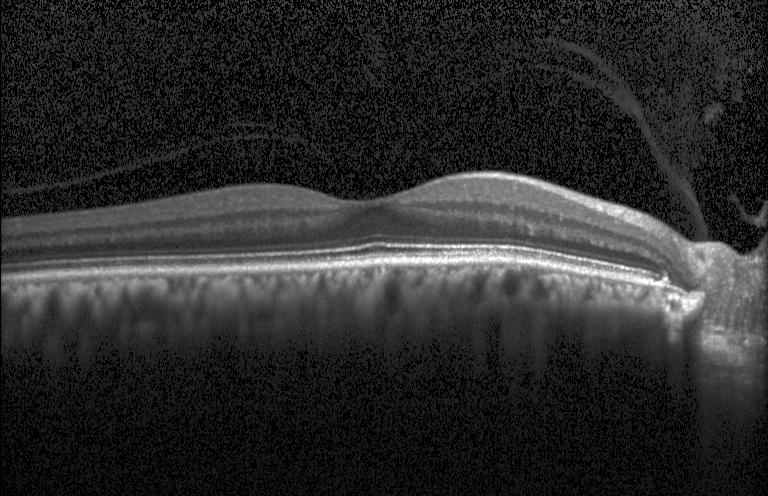

Heidelberg Spectralis, retinal OCT cross-section.
OCT finding: neither choroidal neovascularization, diabetic macular edema, nor drusen.